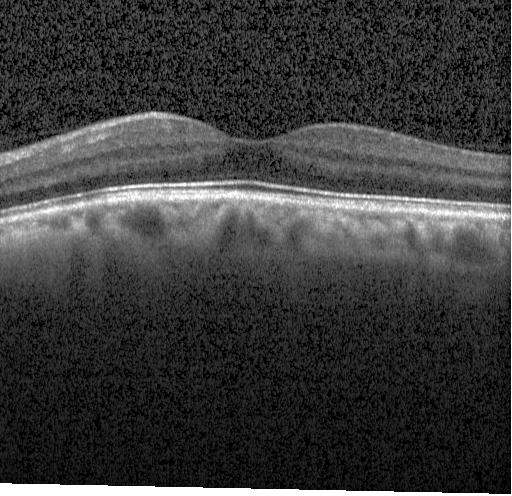 Optical coherence tomography scan. Impression: no evidence of choroidal neovascularization, diabetic macular edema, or drusen.